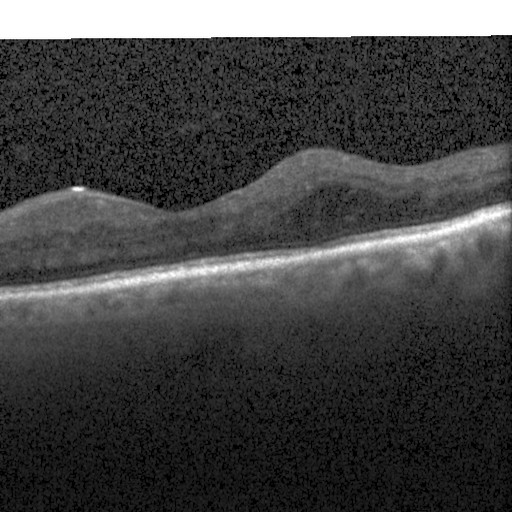

The scan shows diabetic macular edema.